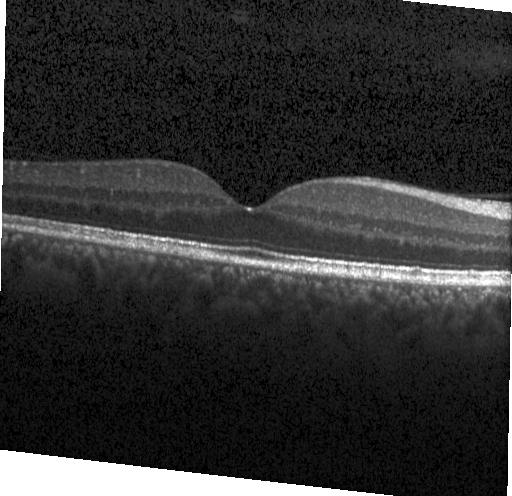
The scan shows no CNV, no DME, and no drusen.